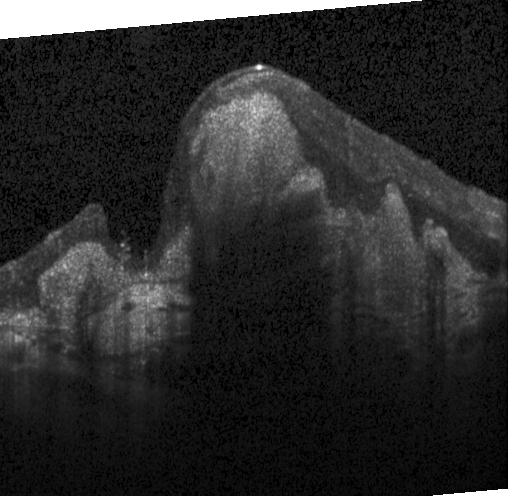
Spectral-domain optical coherence tomography. Horizontal scan through the fovea. OCT line scan
The scan shows choroidal neovascularization (CNV).